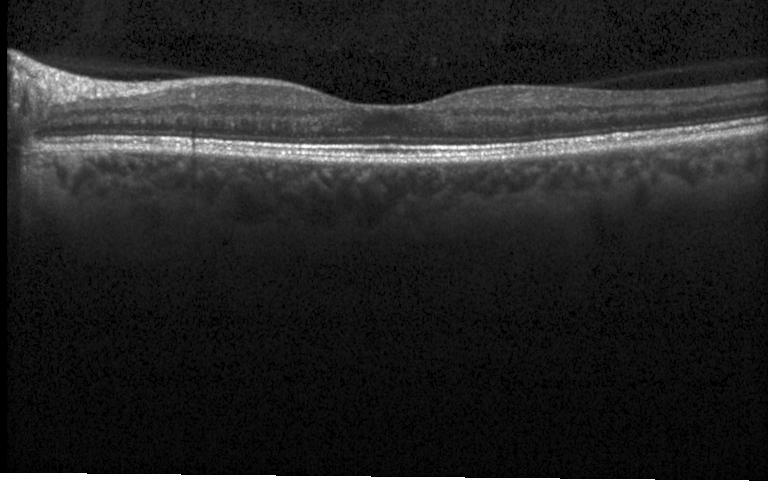

The scan shows no evidence of choroidal neovascularization, diabetic macular edema, or drusen.